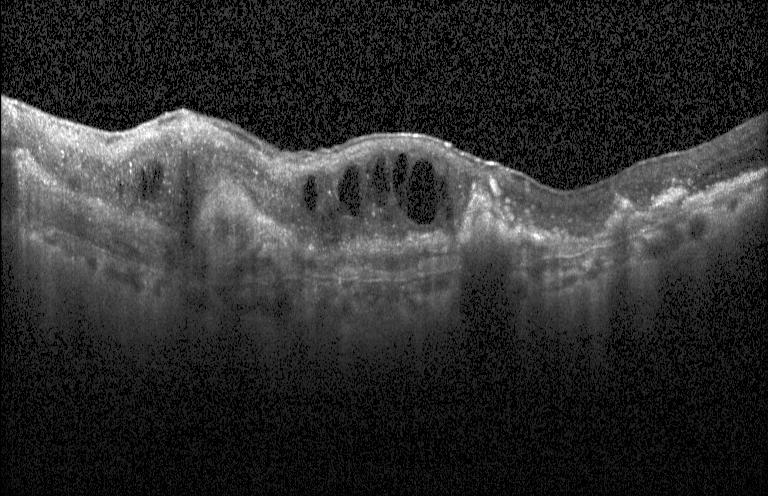

Retinal OCT B-scan, spectral-domain optical coherence tomography. Impression: a choroidal neovascular membrane.